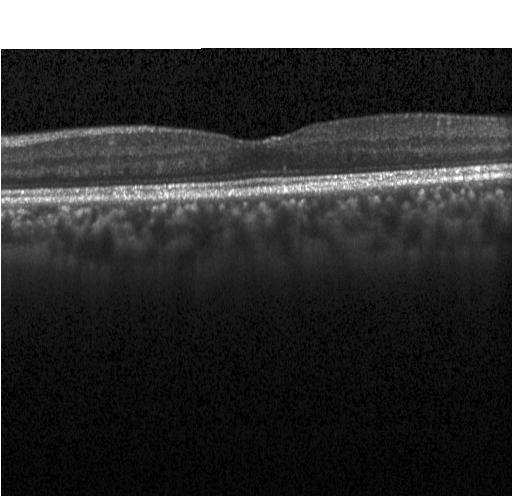
OCT line scan. Heidelberg Spectralis — Macular OCT: neither choroidal neovascularization, diabetic macular edema, nor drusen.